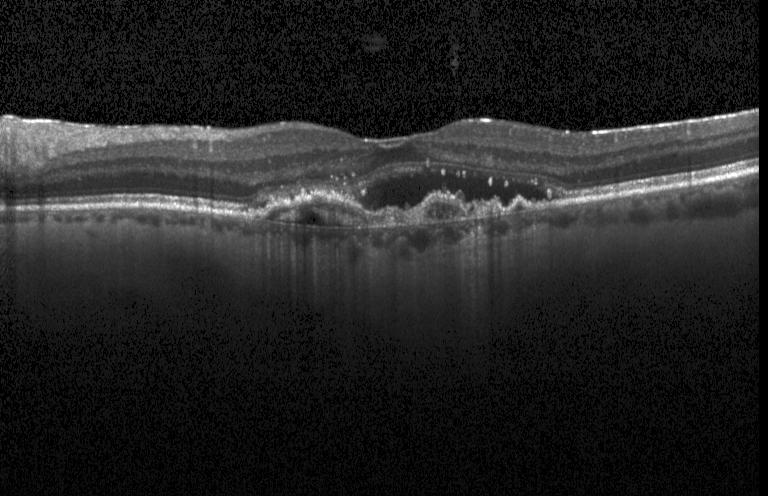
Choroidal neovascularization (CNV).